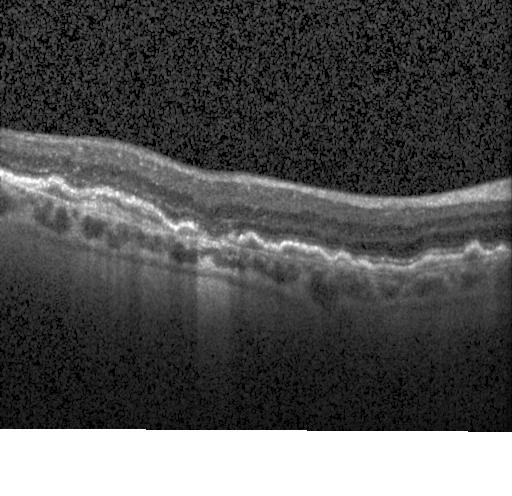 Finding: choroidal neovascularization.